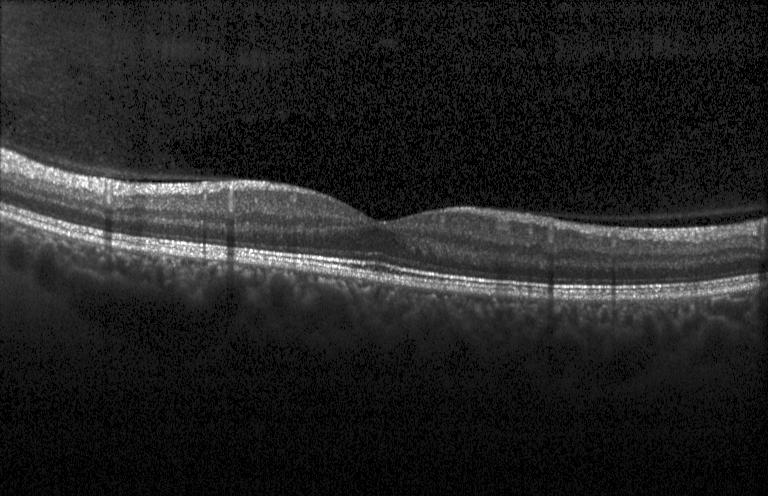 Macular scan · optical coherence tomography B-scan · spectral-domain optical coherence tomography · acquired on a Heidelberg Spectralis.
Assessment: no choroidal neovascularization, no diabetic macular edema, and no drusen.